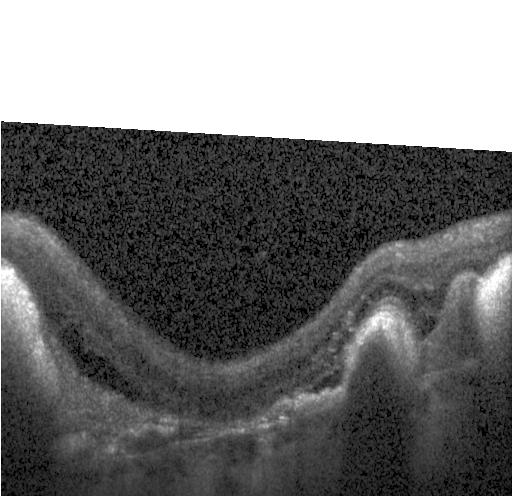

Diagnosis: a choroidal neovascular membrane.